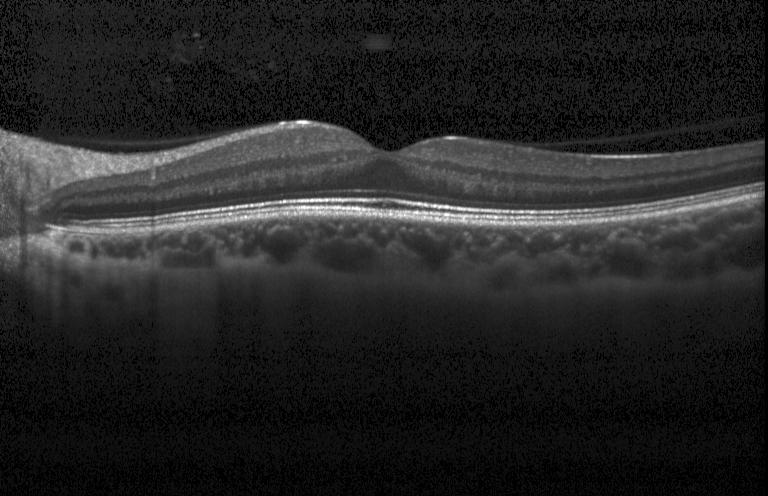
OCT line scan. No choroidal neovascularization, no diabetic macular edema, and no drusen.